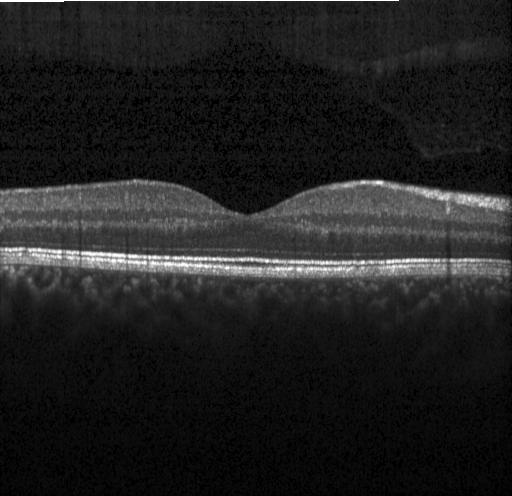 Diagnosis: no evidence of choroidal neovascularization, diabetic macular edema, or drusen.